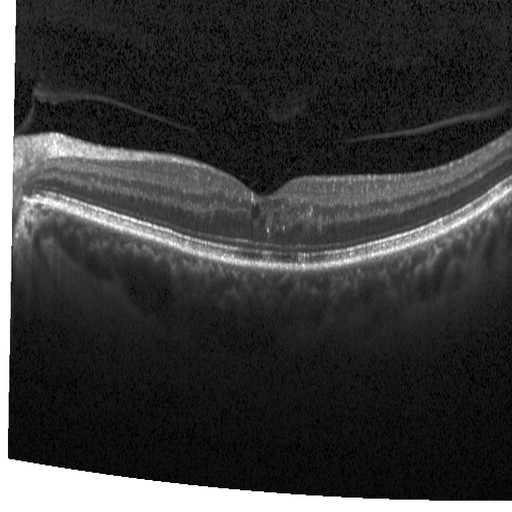

OCT scan showing diabetic macular edema.